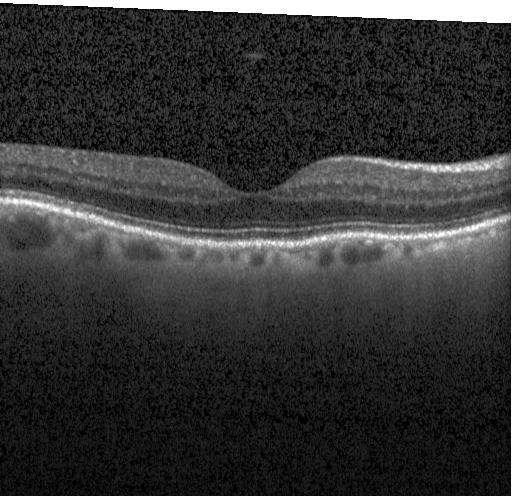 Instrument: Heidelberg Spectralis · SD-OCT · retinal OCT cross-section. Diagnosis: no choroidal neovascularization, diabetic macular edema, or drusen.